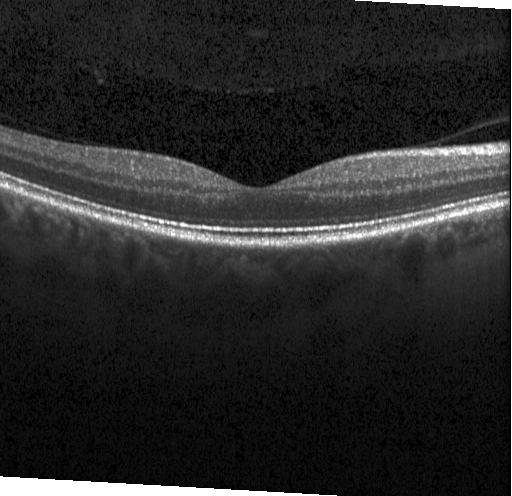

Spectral-domain optical coherence tomography. Horizontal scan through the fovea. Retinal OCT B-scan. Acquired on a Heidelberg Spectralis. Finding: no CNV, no DME, and no drusen.